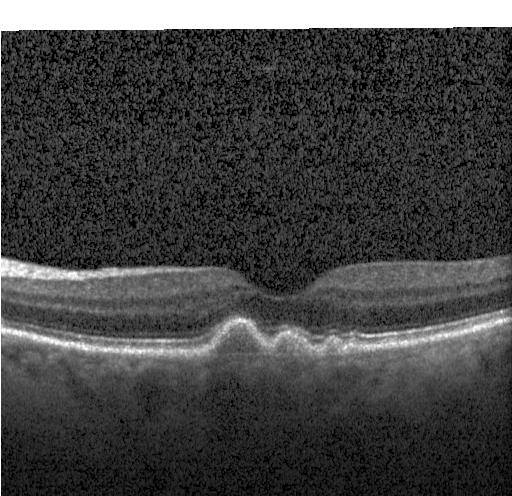 SD-OCT · OCT B-scan · instrument: Heidelberg Spectralis — The scan shows multiple drusen.